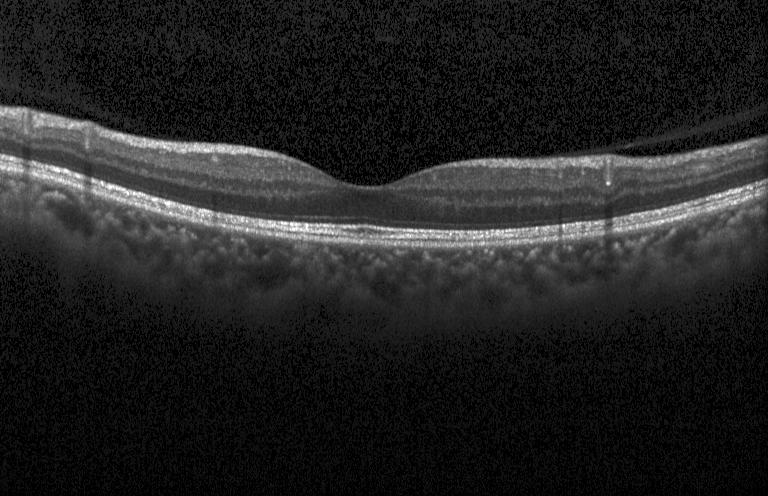 OCT B-scan.
Finding: no choroidal neovascularization, no diabetic macular edema, and no drusen.